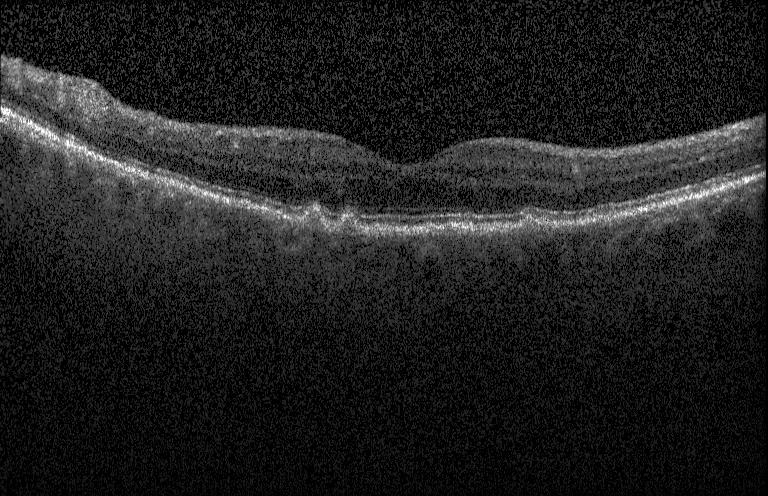 Optical coherence tomography B-scan, SD-OCT.
Dx: sub-RPE drusenoid deposits.